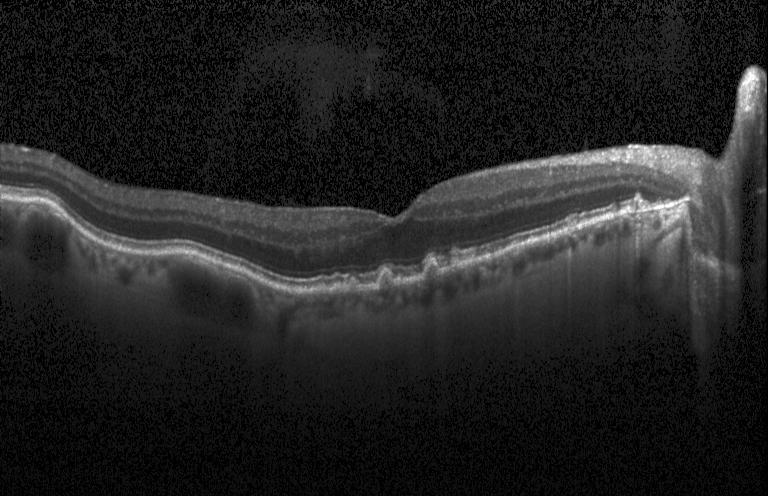

OCT B-scan showing multiple drusen.